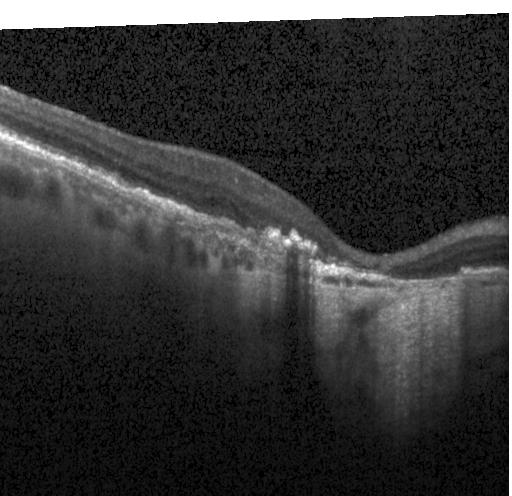

Optical coherence tomography scan.
Dx: choroidal neovascularization (CNV).